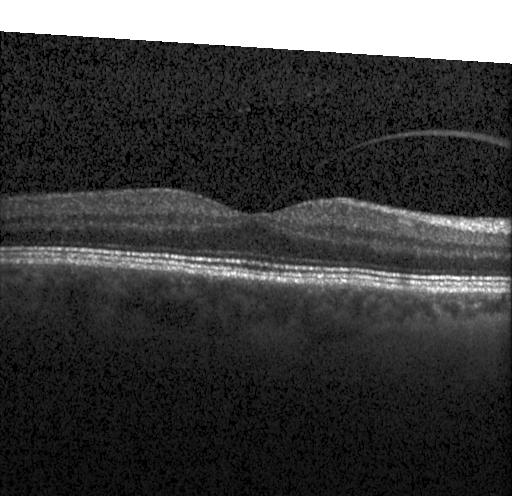
OCT B-scan · fovea-centered · spectral-domain OCT.
Dx: no choroidal neovascularization, no diabetic macular edema, and no drusen.